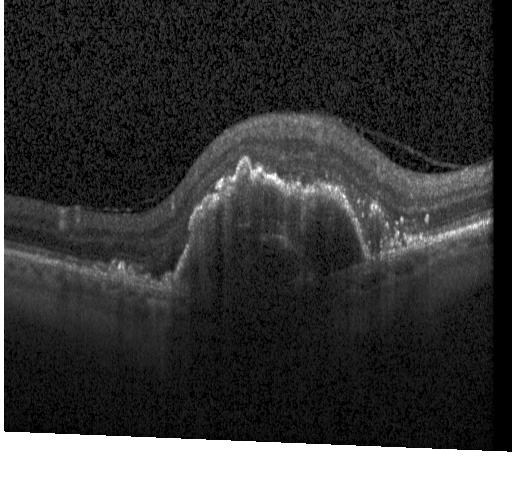

Spectral-domain optical coherence tomography; retinal OCT cross-section. Finding: a choroidal neovascular membrane.